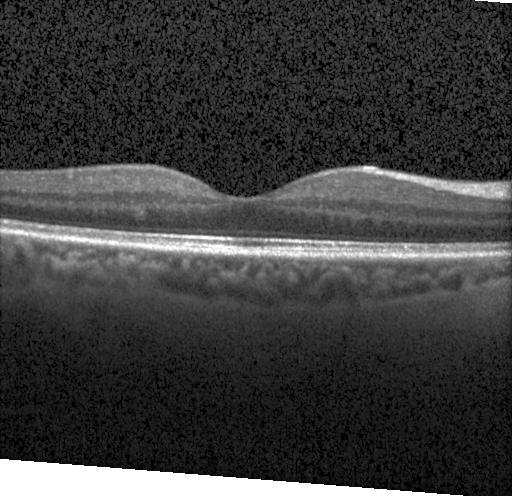 OCT scan showing no evidence of choroidal neovascularization, diabetic macular edema, or drusen.